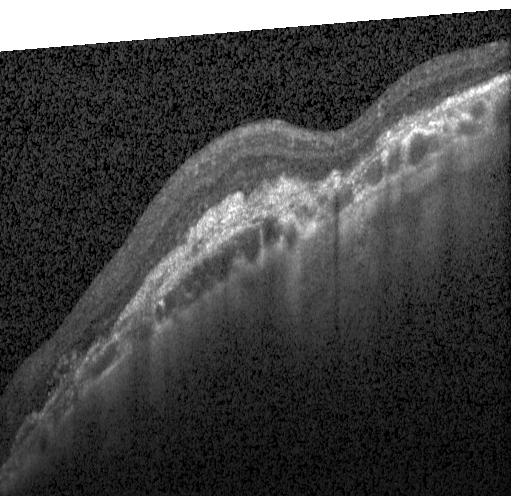

Optical coherence tomography B-scan; instrument: Heidelberg Spectralis; centered on the fovea
Diagnosis: a choroidal neovascular membrane.